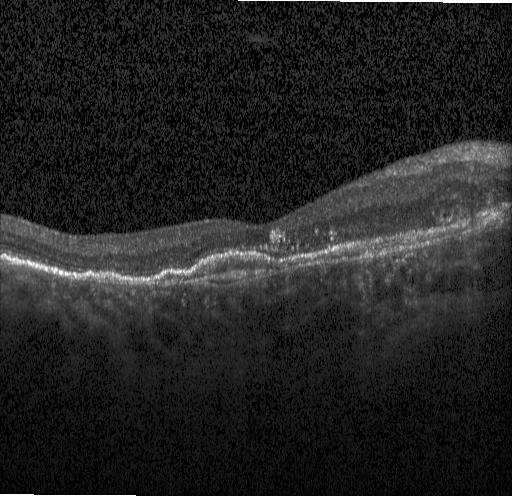
Macular scan; retinal OCT B-scan; instrument: Heidelberg Spectralis; spectral-domain OCT — This B-scan demonstrates a choroidal neovascular membrane.